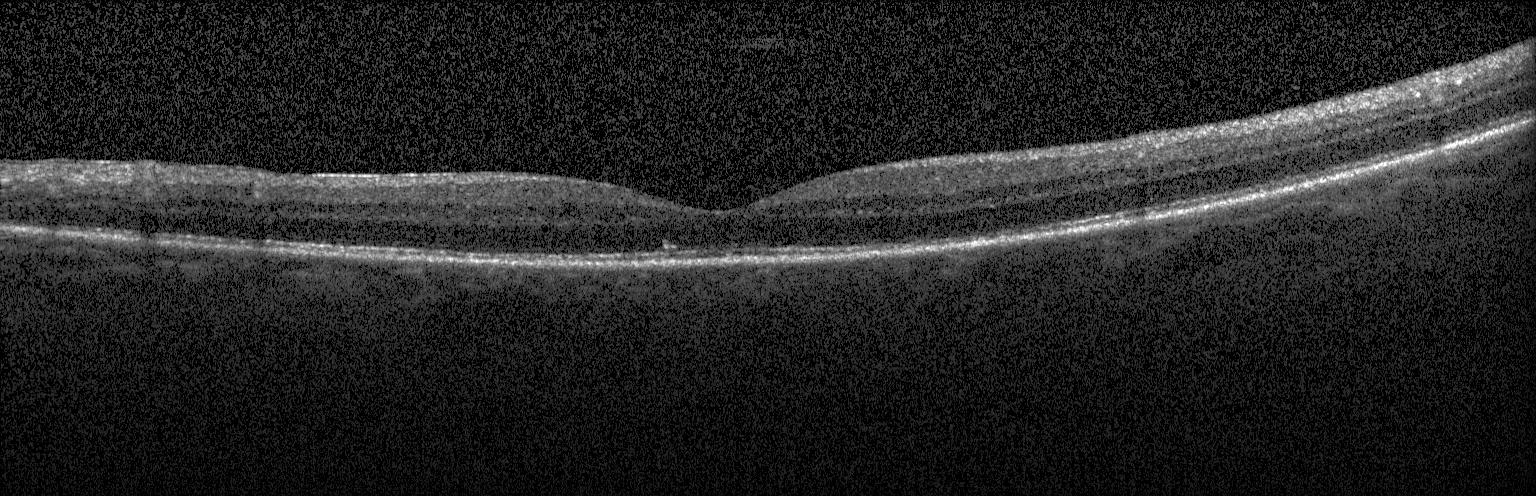 OCT line scan. Dx: neither choroidal neovascularization, diabetic macular edema, nor drusen.